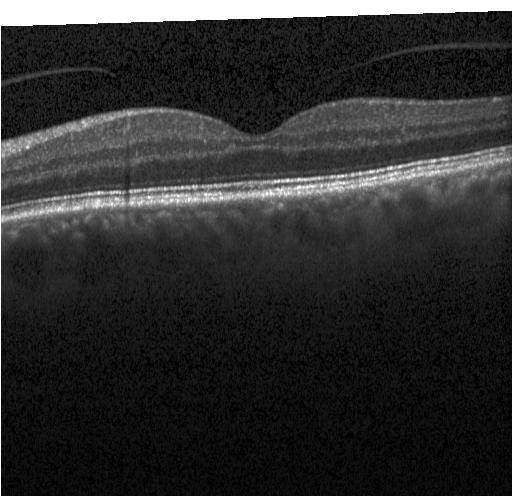
Diagnosis: neither choroidal neovascularization, diabetic macular edema, nor drusen.